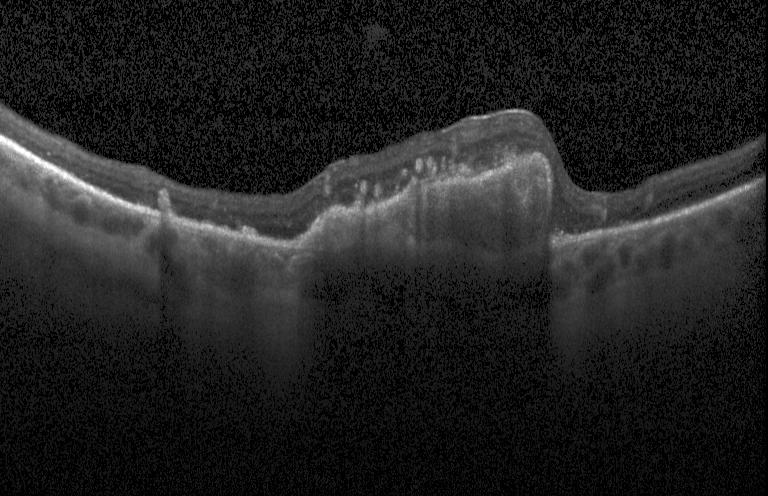 Dx: CNV.